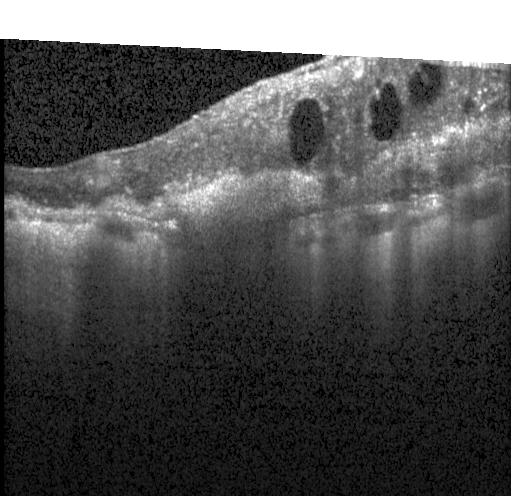

Acquired on a Heidelberg Spectralis; horizontal scan through the fovea; retinal OCT cross-section — Macular OCT: choroidal neovascularization (CNV).